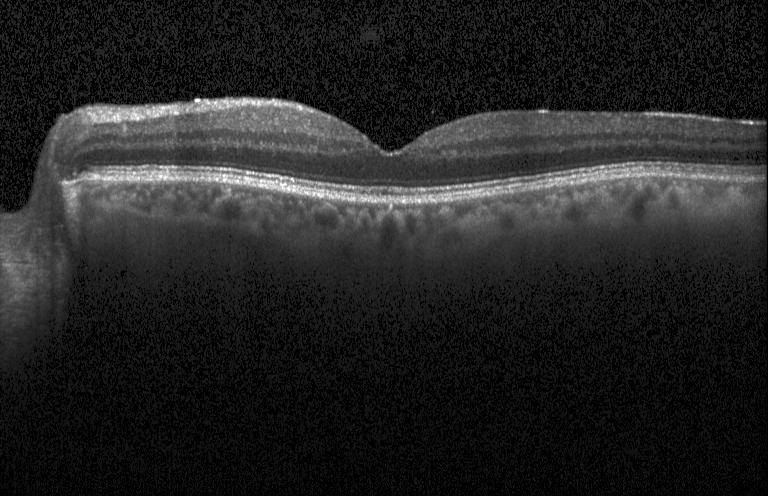

Through the macula. Retinal OCT cross-section. Spectral-domain optical coherence tomography. Heidelberg Spectralis
No evidence of CNV, DME, or drusen.